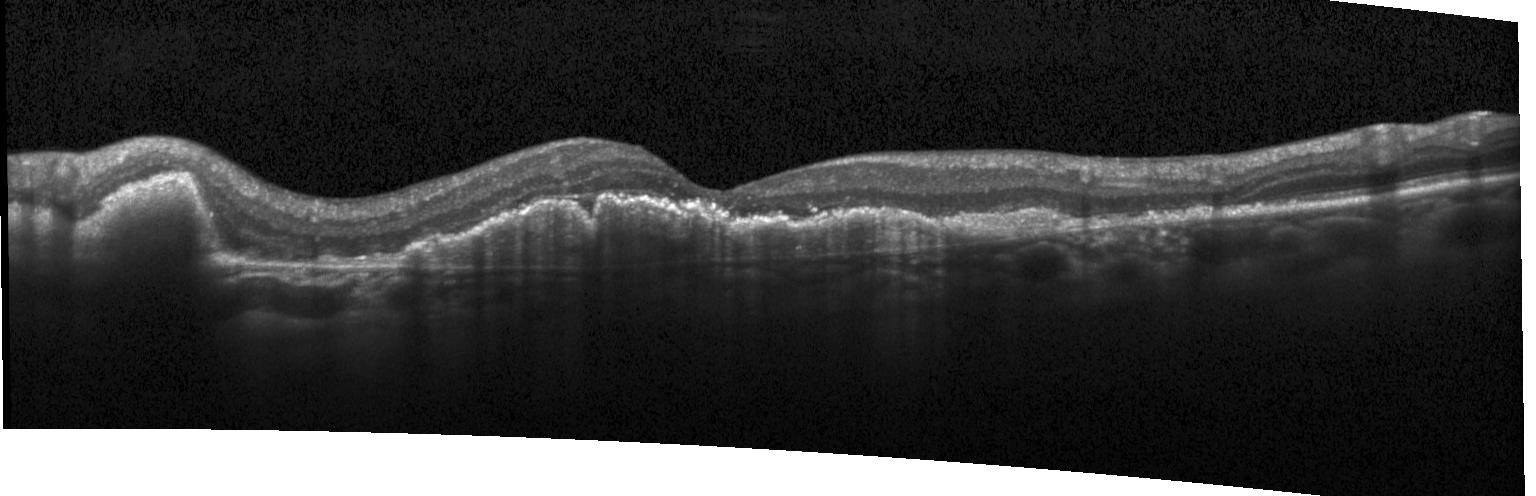 Optical coherence tomography B-scan; horizontal scan through the fovea. Diagnosis: CNV.